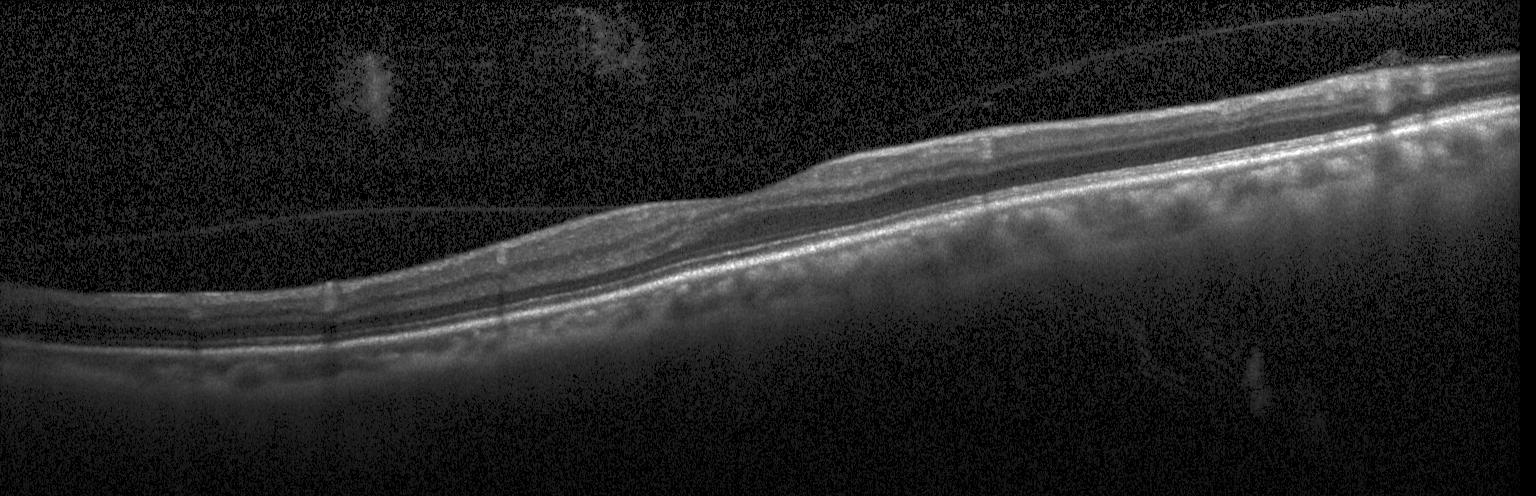 Finding: no choroidal neovascularization, diabetic macular edema, or drusen.